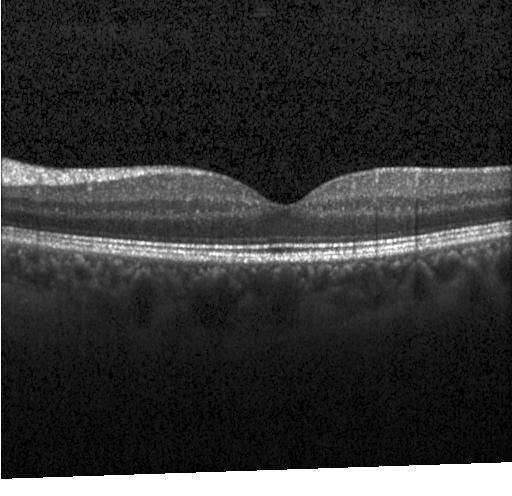

Diagnosis: no choroidal neovascularization, no diabetic macular edema, and no drusen.